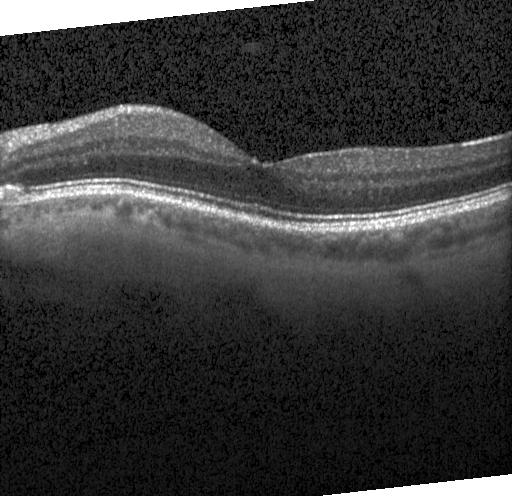

Spectral-domain OCT B-scan: multiple drusen.